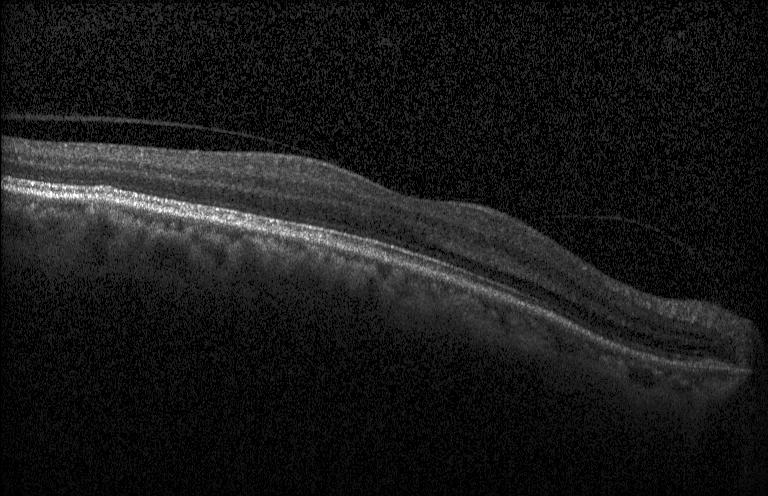 Retinal OCT cross-section. Dx: neither choroidal neovascularization, diabetic macular edema, nor drusen.